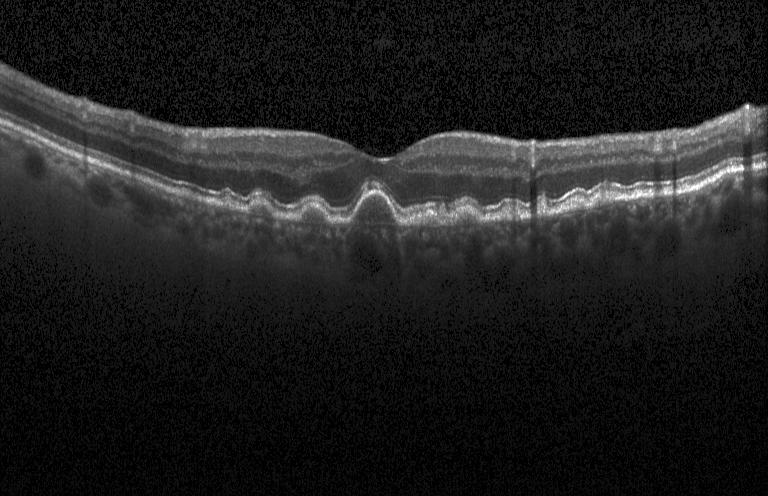
OCT B-scan; SD-OCT
Finding: sub-RPE drusenoid deposits.